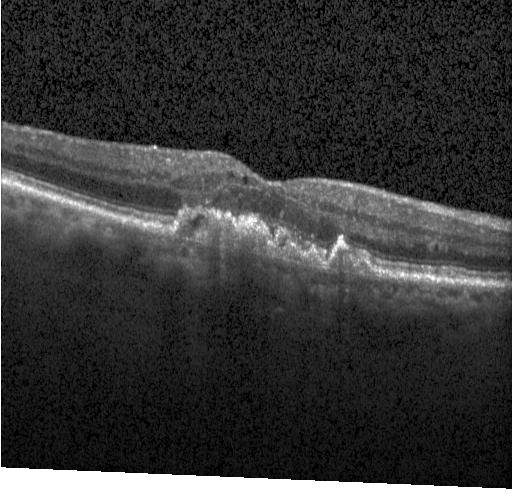

Heidelberg Spectralis · OCT B-scan · macular scan · SD-OCT.
This B-scan demonstrates a choroidal neovascular membrane.